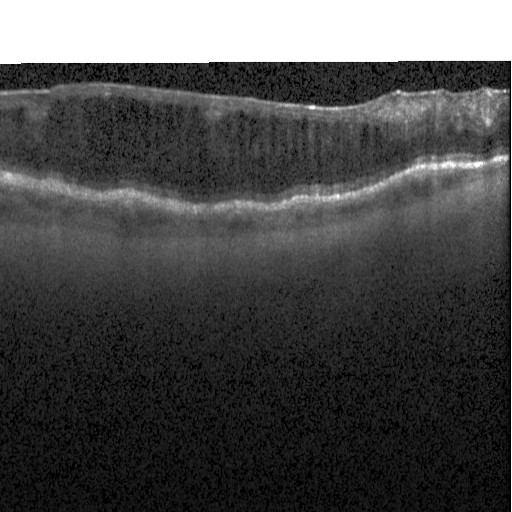

OCT B-scan showing DME.